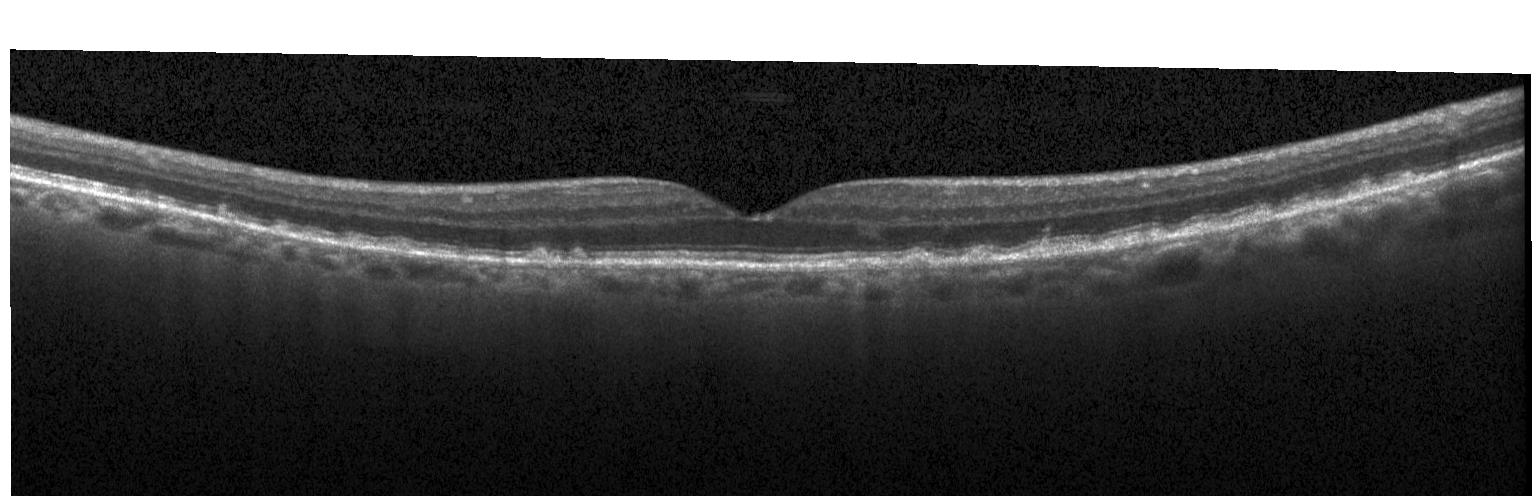

Spectral-domain optical coherence tomography; acquired on a Heidelberg Spectralis; OCT line scan. The scan shows drusen.